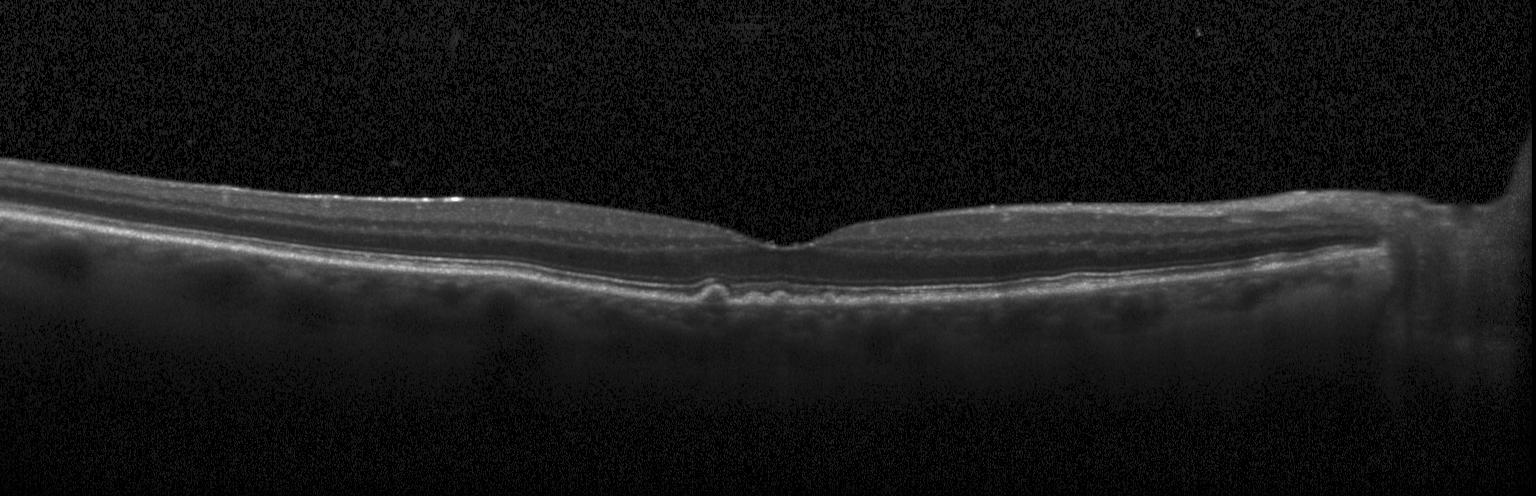
Through the macula, spectral-domain optical coherence tomography, Heidelberg Spectralis OCT system, OCT B-scan — Finding: sub-RPE drusenoid deposits.